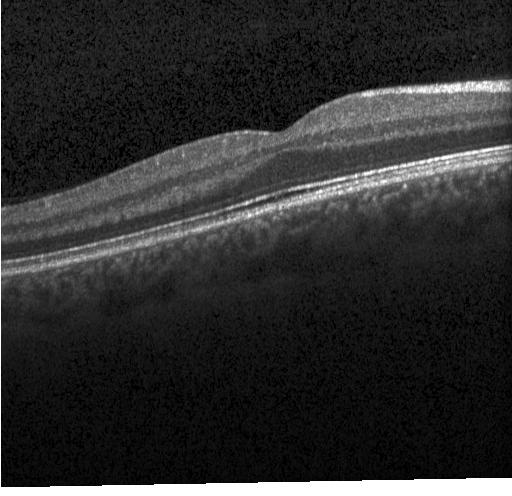
This B-scan demonstrates neither choroidal neovascularization, diabetic macular edema, nor drusen.